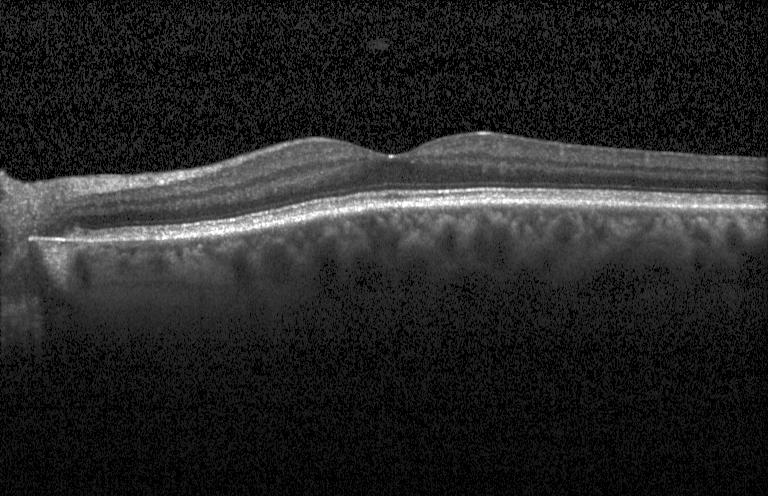

Assessment: neither choroidal neovascularization, diabetic macular edema, nor drusen.